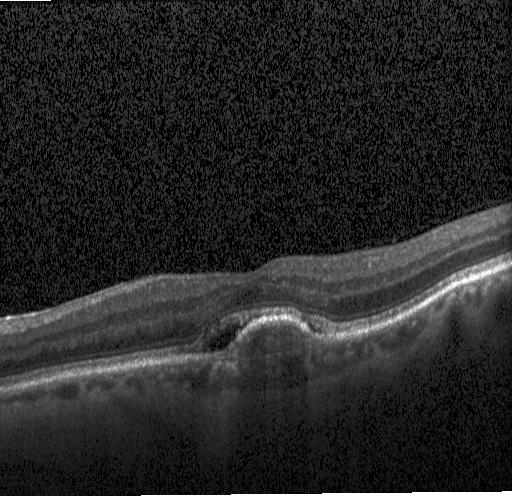
OCT B-scan · fovea-centered · Heidelberg Spectralis · SD-OCT — Macular OCT: choroidal neovascularization.